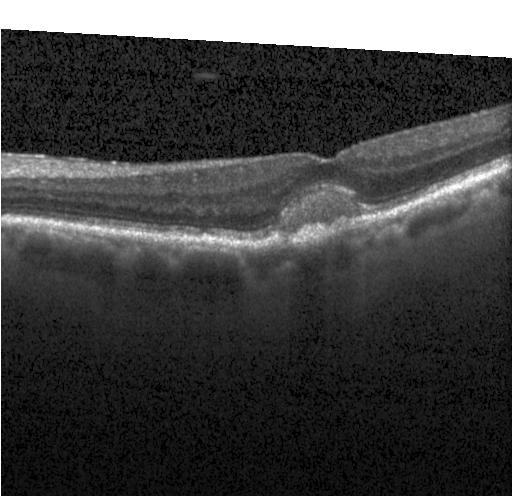 Macular OCT: CNV.